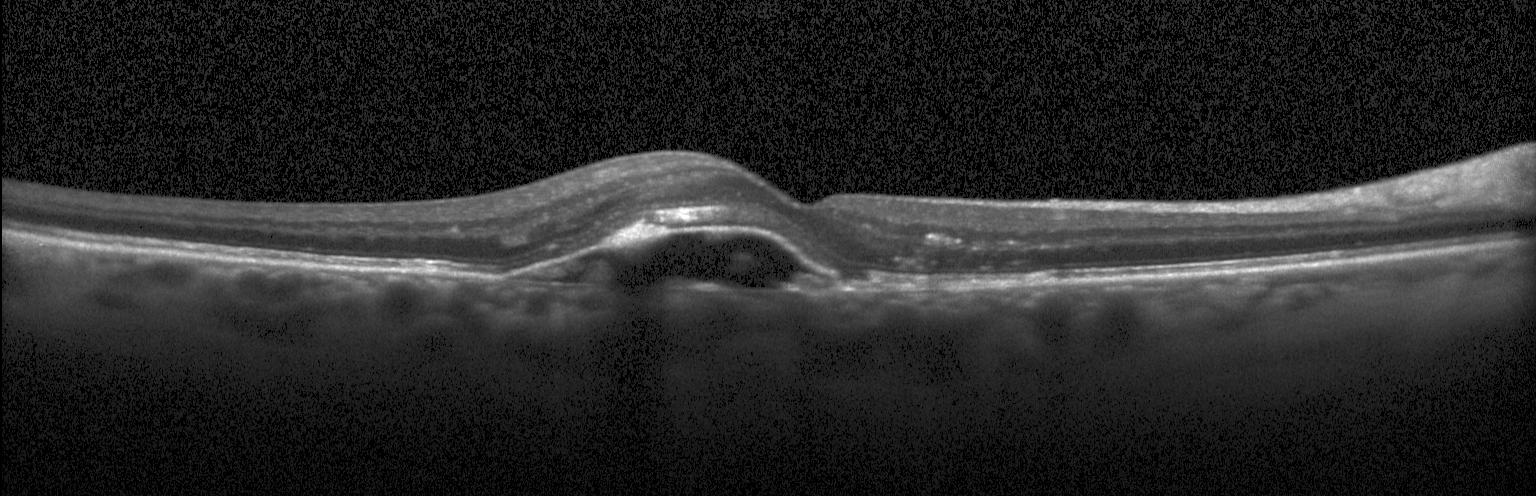

Spectral-domain OCT; centered on the fovea; optical coherence tomography B-scan; Heidelberg Spectralis. Impression: a choroidal neovascular membrane.